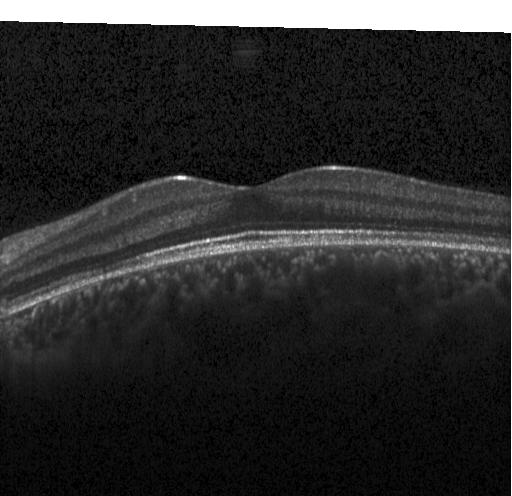

Retinal OCT cross-section; through the macula; instrument: Heidelberg Spectralis; SD-OCT
Diagnosis: no evidence of CNV, DME, or drusen.